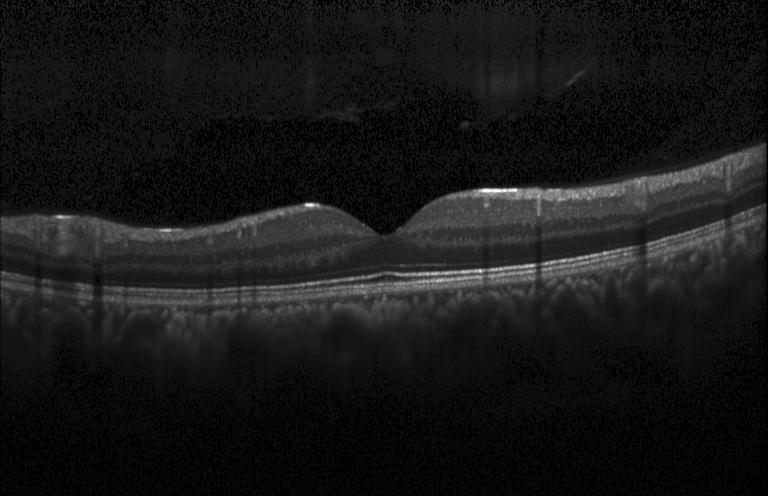
Optical coherence tomography scan — Impression: no evidence of choroidal neovascularization, diabetic macular edema, or drusen.